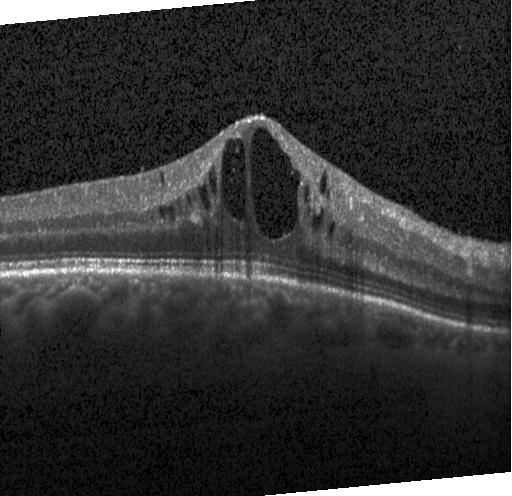 SD-OCT, OCT line scan.
Assessment: diabetic macular edema.